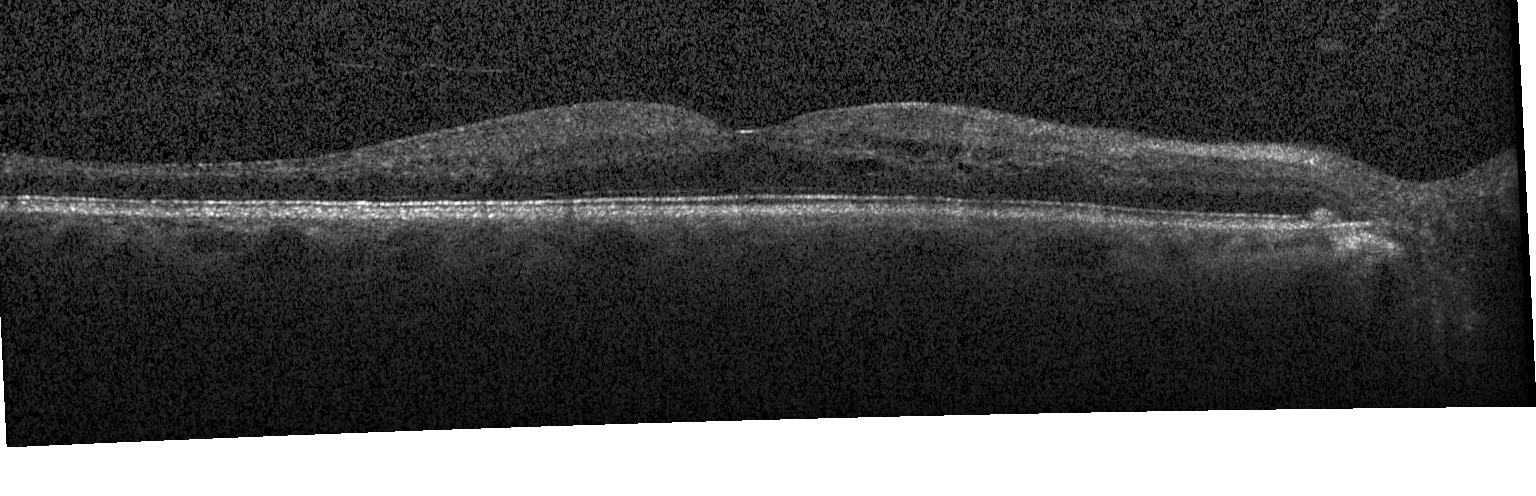

Dx: diabetic macular edema.